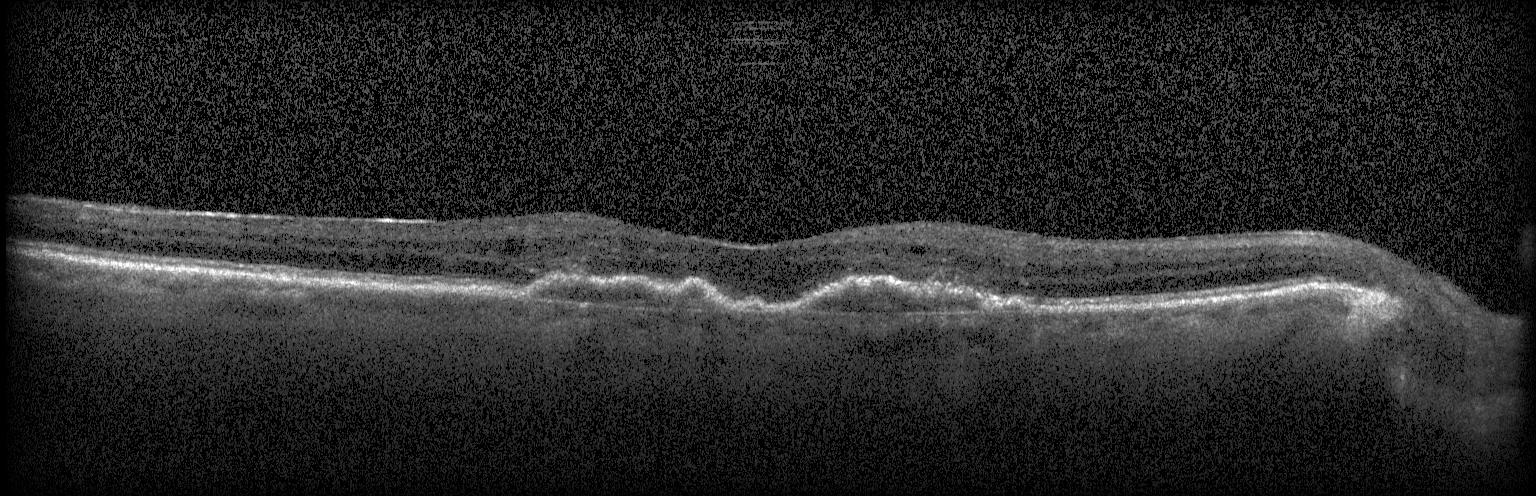

Macular OCT demonstrating a choroidal neovascular membrane.